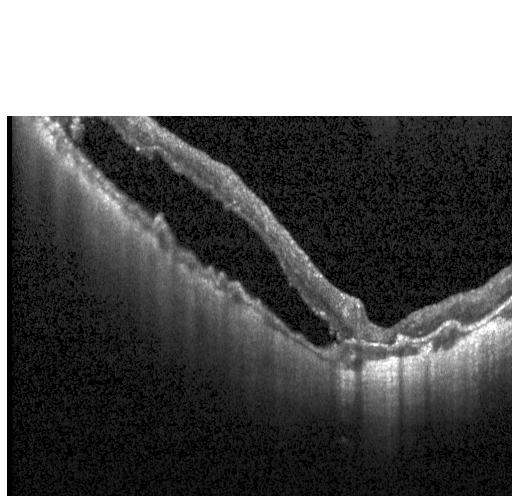
Diagnosis: CNV.